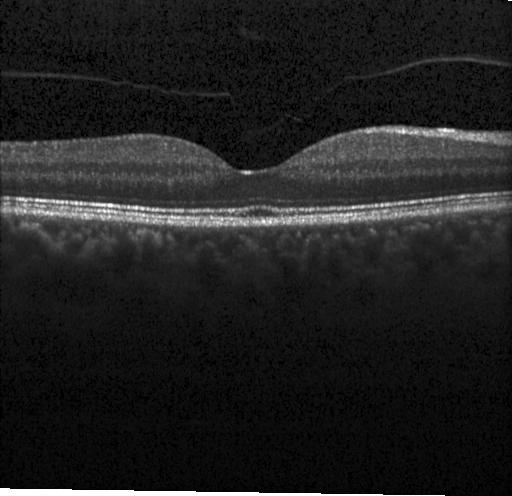

Finding: no evidence of choroidal neovascularization, diabetic macular edema, or drusen.